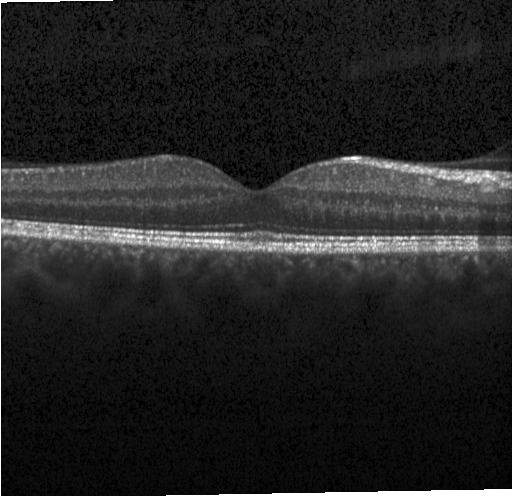

Retinal OCT cross-section; through the macula; Heidelberg Spectralis. Diagnosis: no choroidal neovascularization, diabetic macular edema, or drusen.